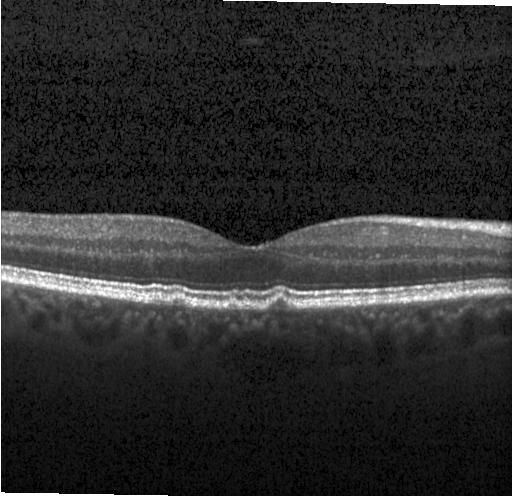
Horizontal scan through the fovea · optical coherence tomography B-scan
Impression: multiple drusen.